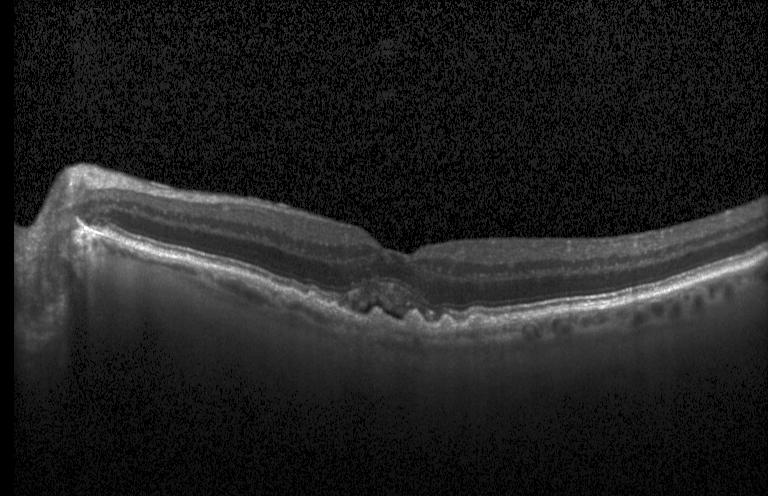 Spectral-domain optical coherence tomography · optical coherence tomography scan · fovea-centered · instrument: Heidelberg Spectralis. The scan shows choroidal neovascularization.